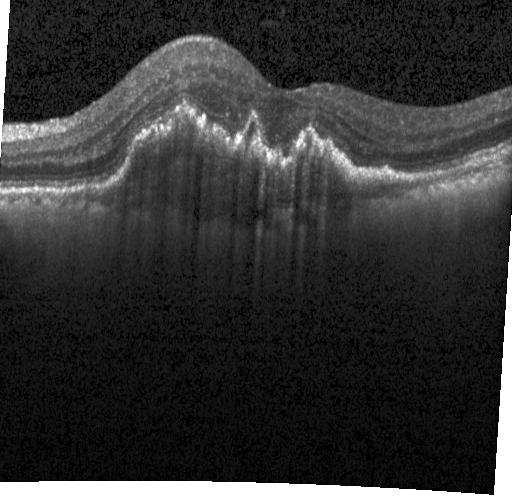

Retinal OCT B-scan
Finding: a choroidal neovascular membrane.